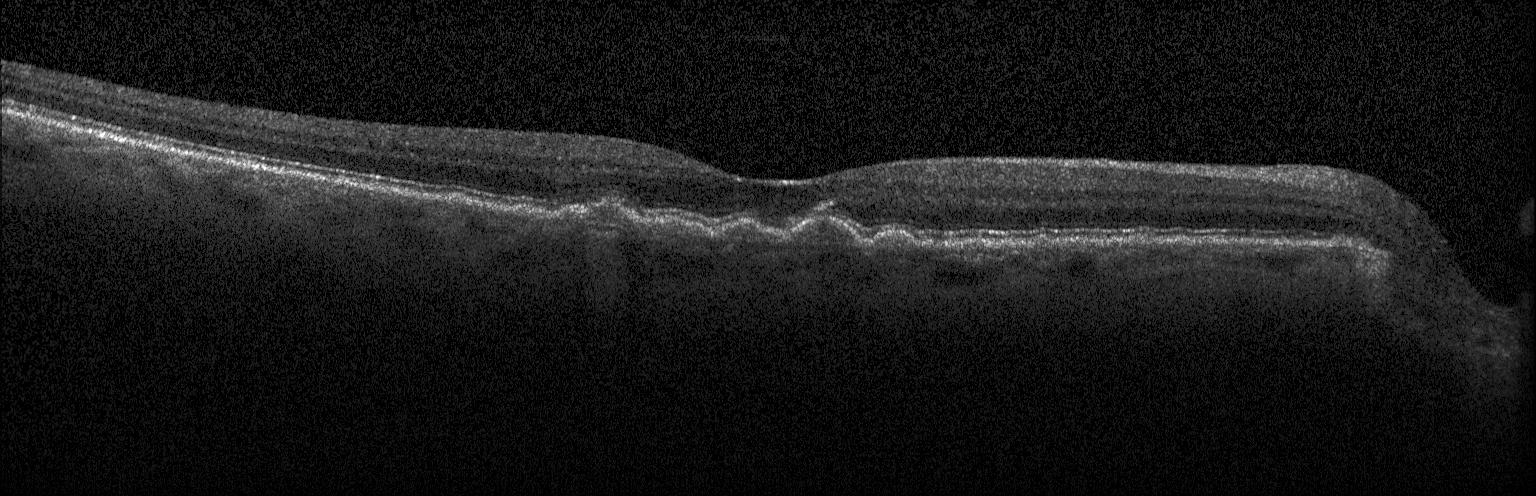
Retinal OCT B-scan, Heidelberg Spectralis, spectral-domain OCT — Sub-RPE drusenoid deposits.